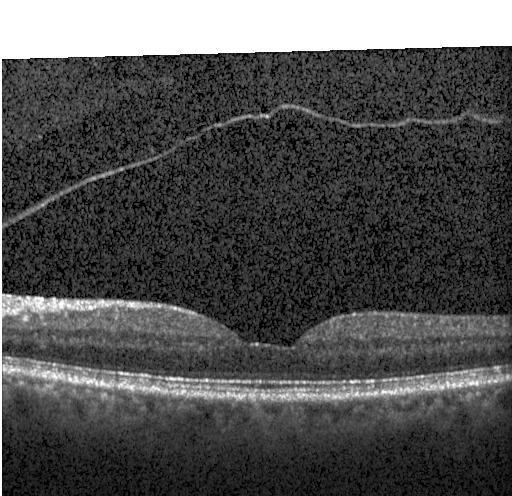 Retinal OCT cross-section showing no evidence of CNV, DME, or drusen.